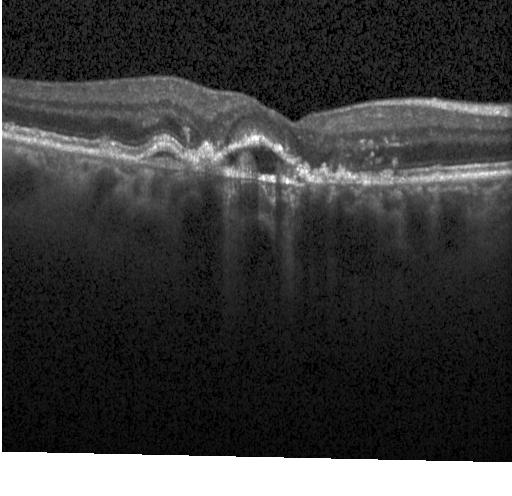 Instrument: Heidelberg Spectralis. Retinal OCT cross-section. Spectral-domain optical coherence tomography.
This B-scan demonstrates choroidal neovascularization (CNV).